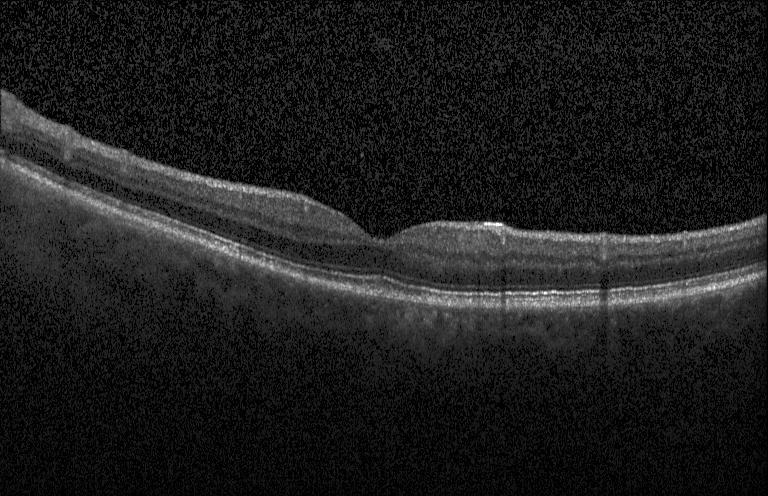
Dx: no choroidal neovascularization, no diabetic macular edema, and no drusen.